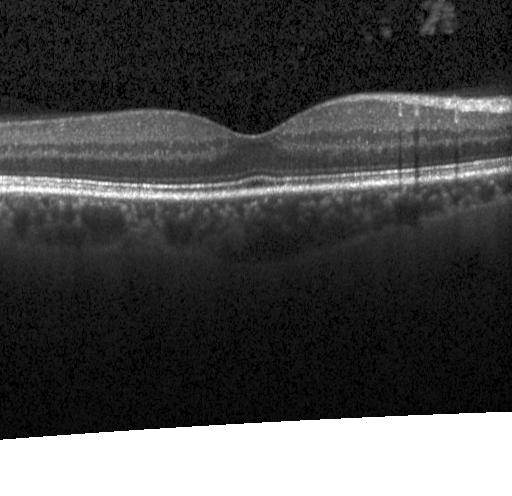 Fovea-centered. Spectral-domain optical coherence tomography. OCT line scan. Instrument: Heidelberg Spectralis.
Finding: no CNV, no DME, and no drusen.